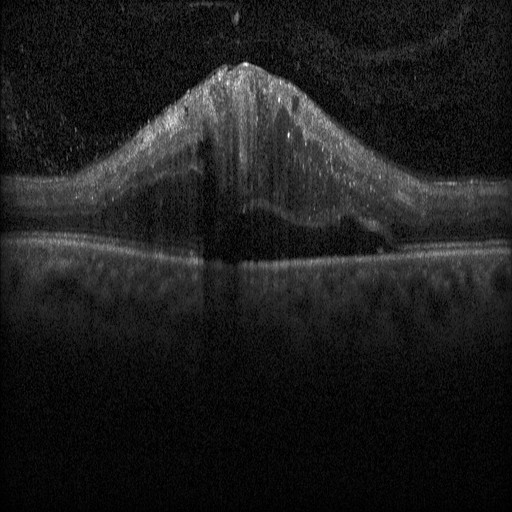 Optical coherence tomography scan — Macular OCT: diabetic macular edema.